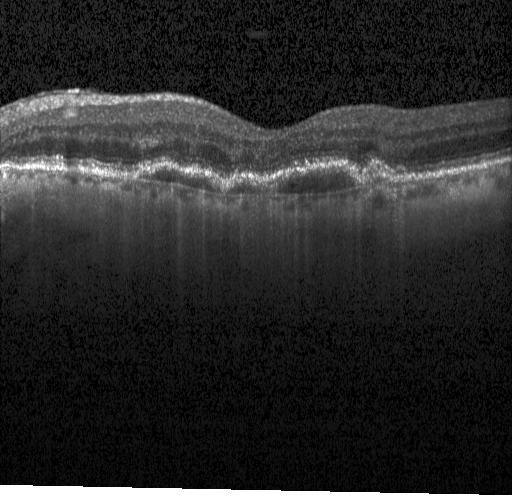 Spectral-domain OCT, optical coherence tomography B-scan, instrument: Heidelberg Spectralis. Impression: CNV.